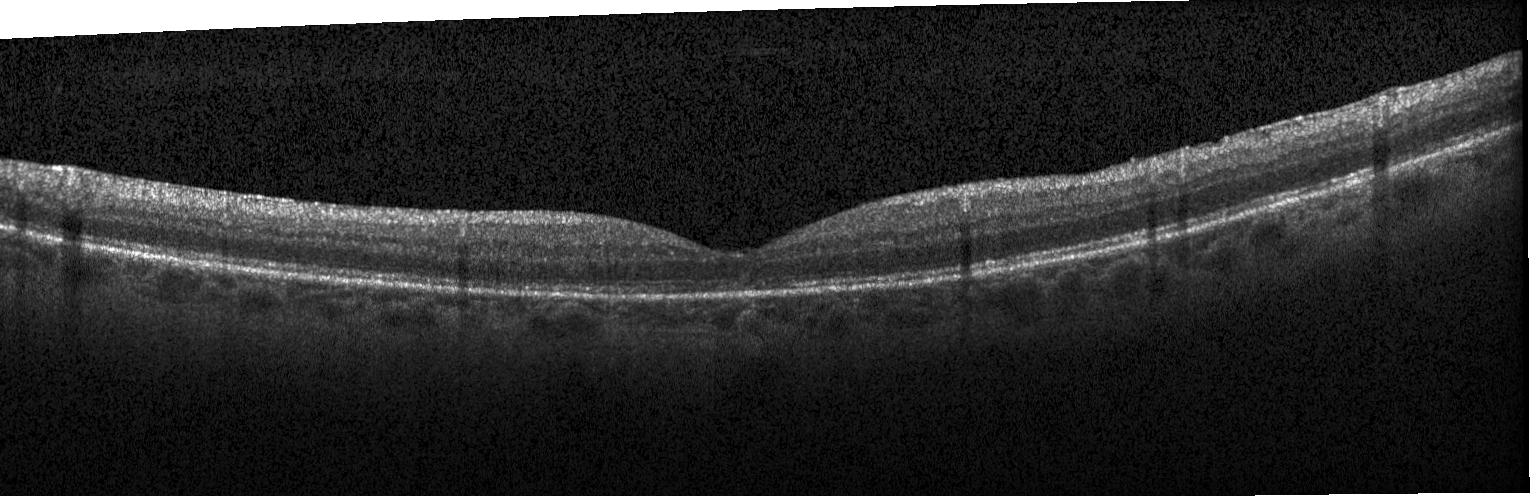 Retinal OCT B-scan
This B-scan demonstrates no evidence of CNV, DME, or drusen.